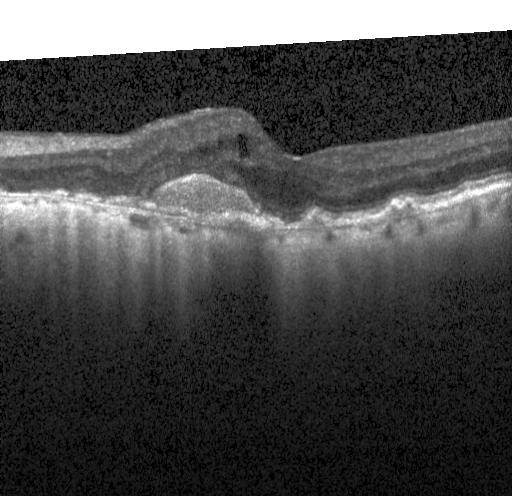

Diagnosis: CNV.